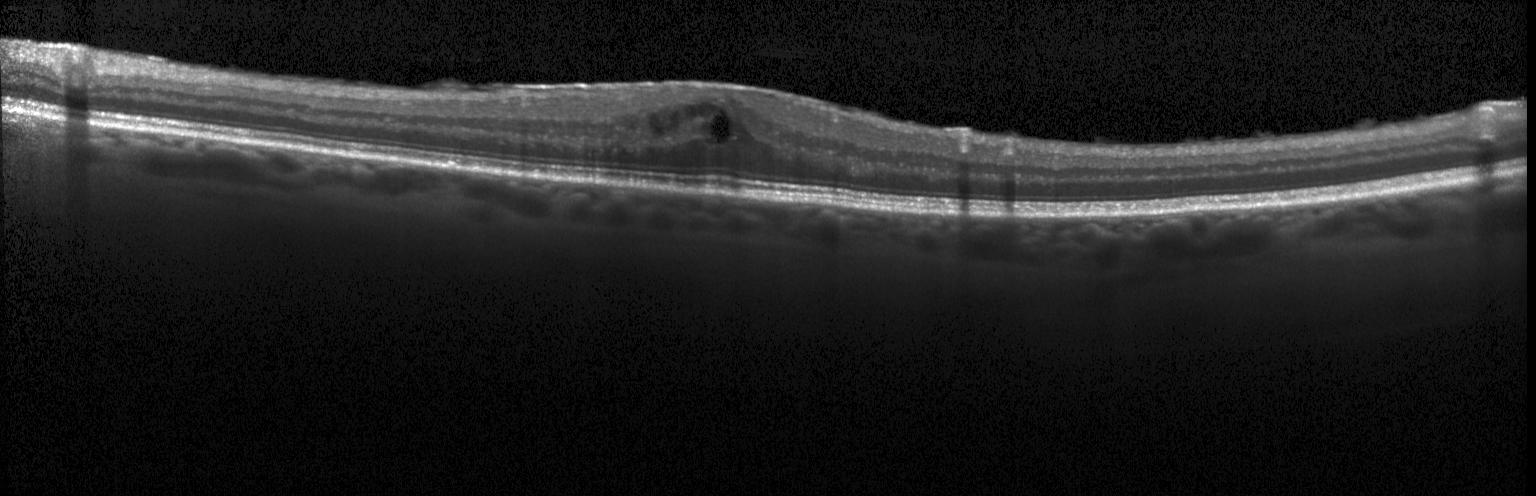
Heidelberg Spectralis. Retinal OCT B-scan. The scan shows DME.